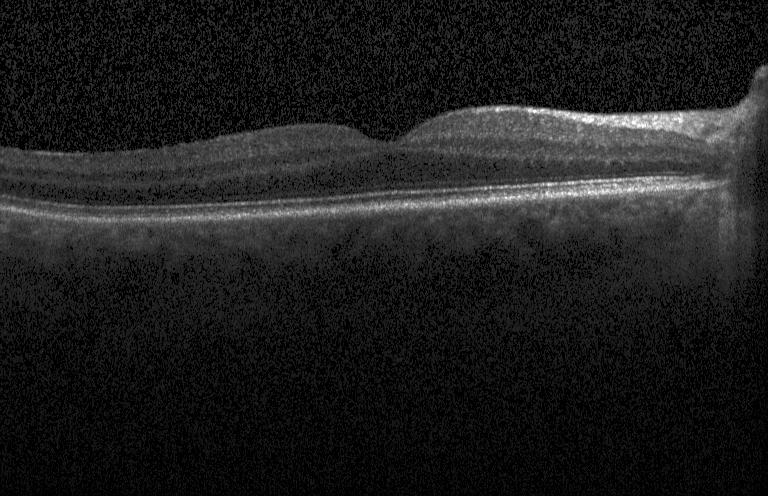 Acquired on a Heidelberg Spectralis · retinal OCT B-scan · fovea-centered — Impression: no choroidal neovascularization, diabetic macular edema, or drusen.